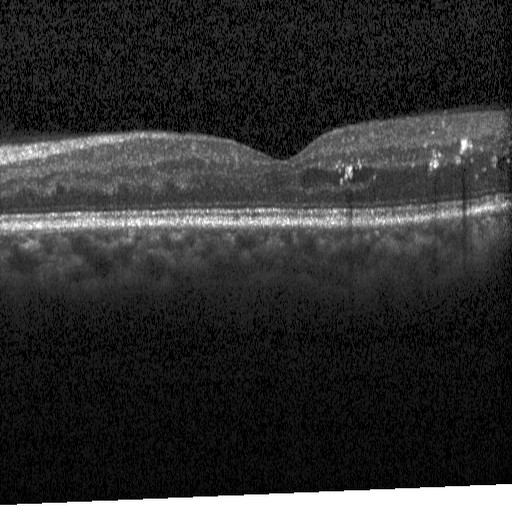 Optical coherence tomography B-scan; Heidelberg Spectralis; macular scan. The scan shows diabetic macular edema.